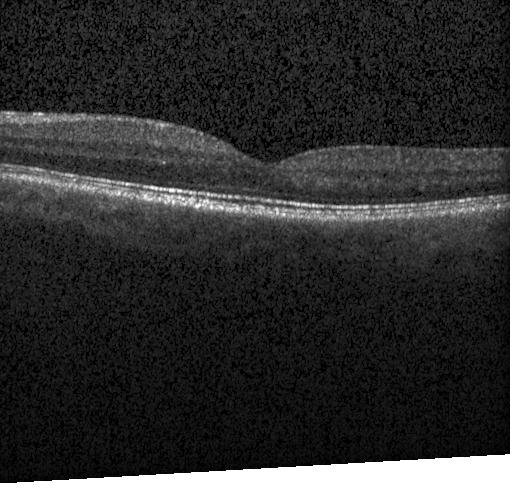 Macular scan · instrument: Heidelberg Spectralis · retinal OCT cross-section · SD-OCT.
Finding: no choroidal neovascularization, diabetic macular edema, or drusen.